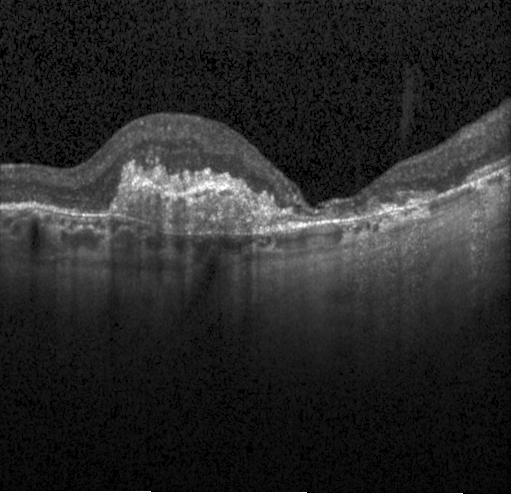

Heidelberg Spectralis OCT system, centered on the fovea, spectral-domain optical coherence tomography, retinal OCT cross-section — Assessment: a choroidal neovascular membrane.